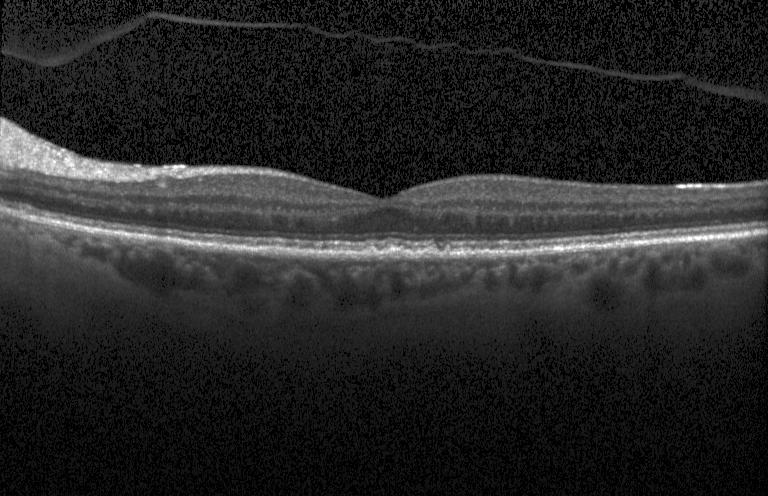

Optical coherence tomography scan · Heidelberg Spectralis · horizontal scan through the fovea — Diagnosis: drusen.